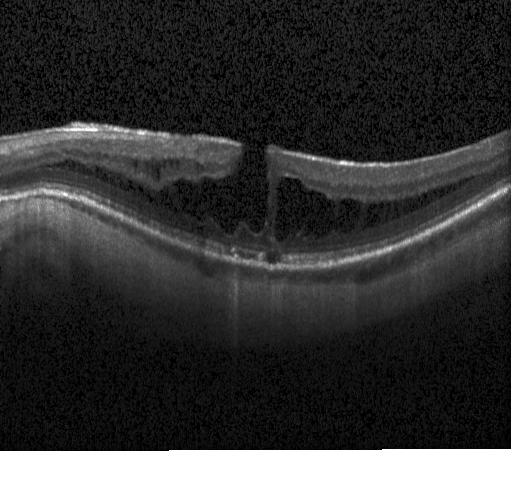

Centered on the fovea, retinal OCT B-scan, SD-OCT.
Finding: diabetic macular edema.